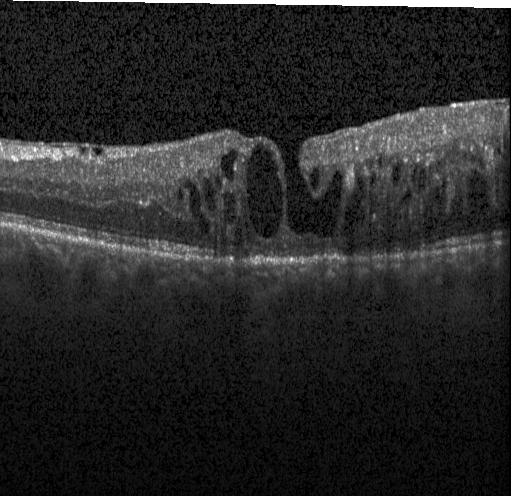
The scan shows diabetic macular edema.